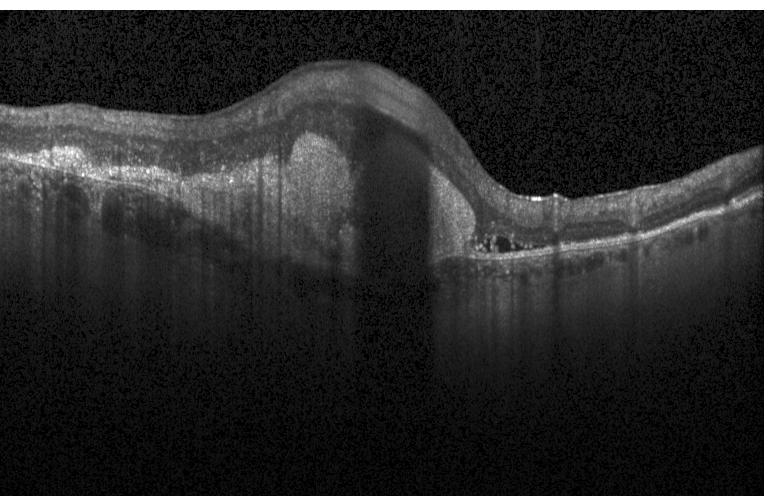

Macular OCT: CNV.